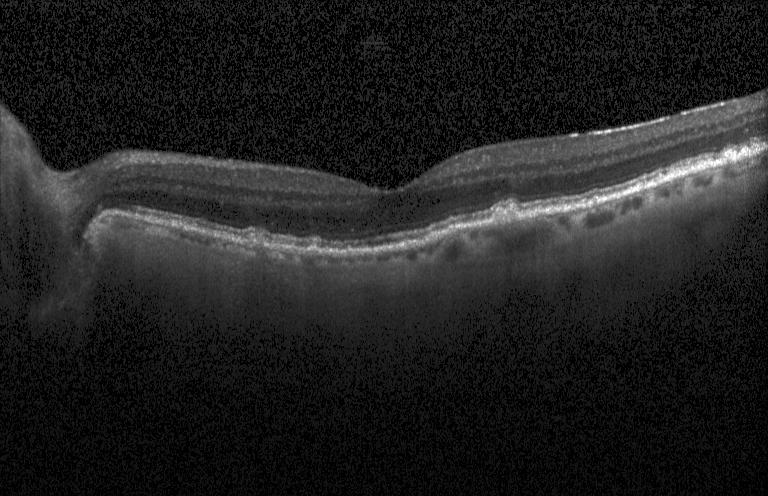
OCT finding: sub-RPE drusenoid deposits.